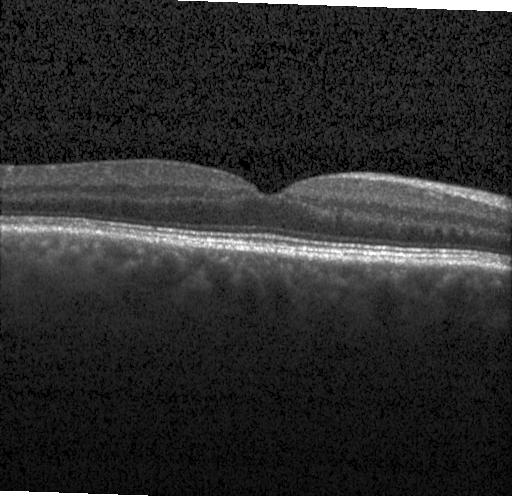

Impression: no evidence of choroidal neovascularization, diabetic macular edema, or drusen.